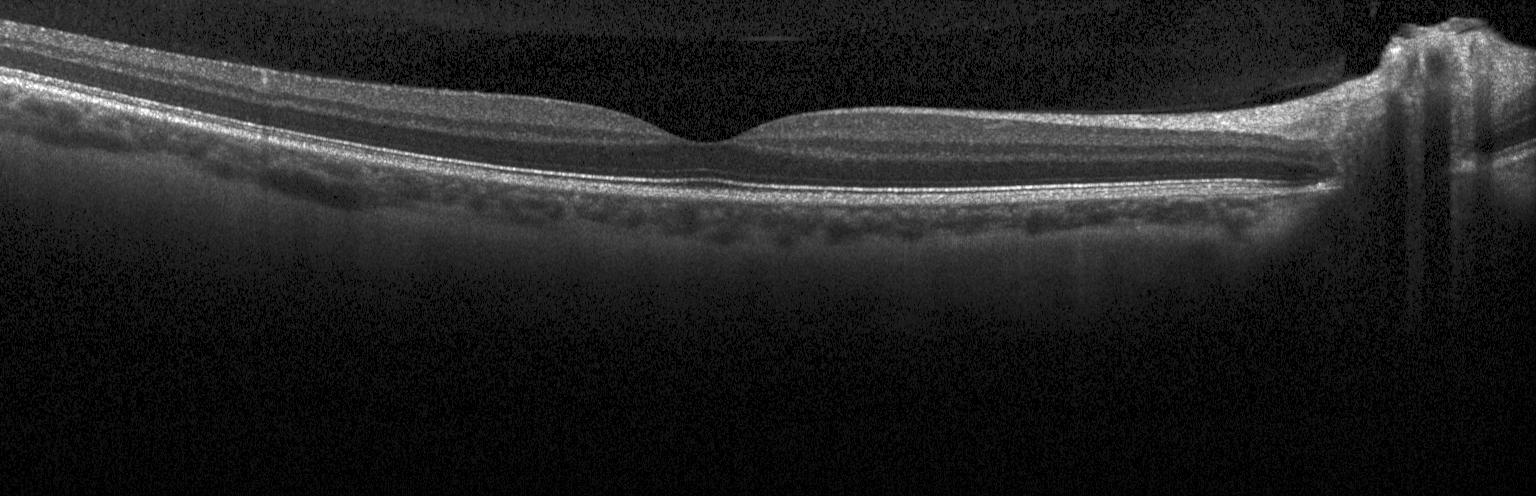
Dx: no choroidal neovascularization, no diabetic macular edema, and no drusen.